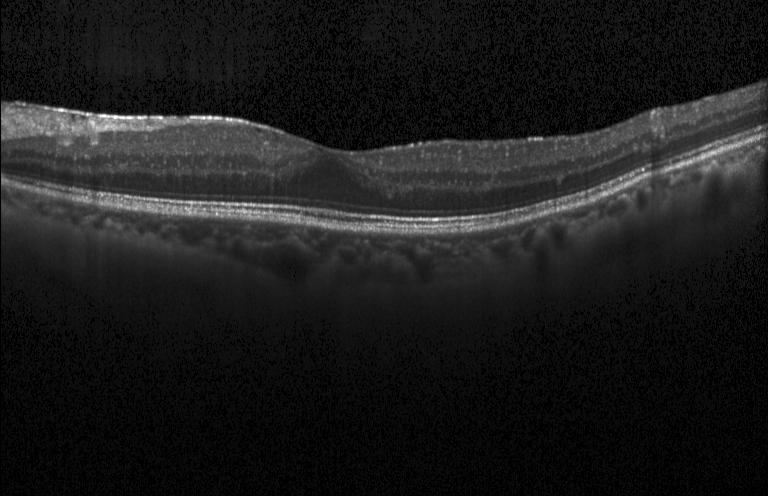 Heidelberg Spectralis, retinal OCT B-scan
Impression: neither choroidal neovascularization, diabetic macular edema, nor drusen.